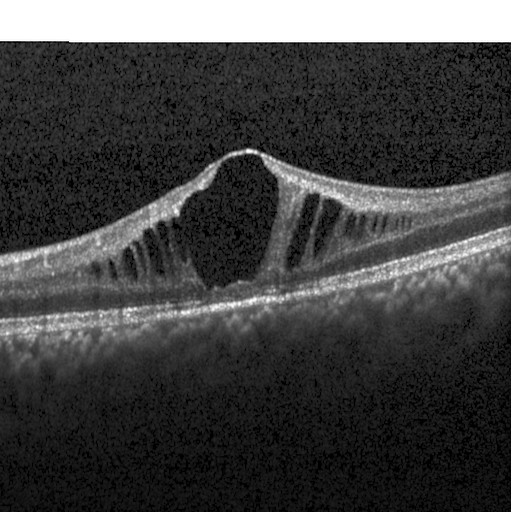

Finding: diabetic macular edema (DME).